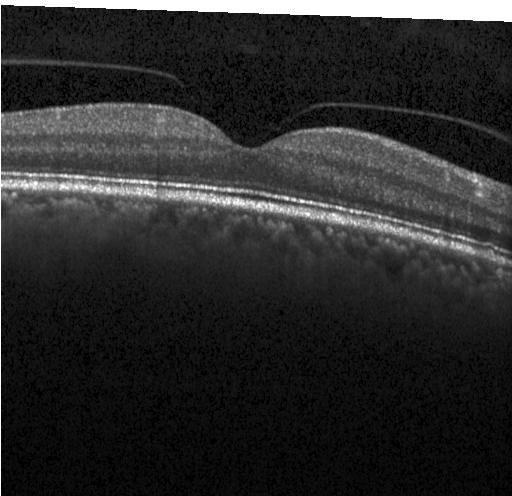 Horizontal scan through the fovea. Retinal OCT B-scan. Diagnosis: neither choroidal neovascularization, diabetic macular edema, nor drusen.